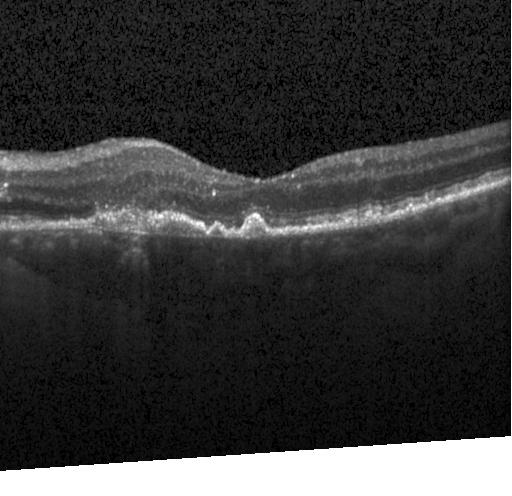
Diagnosis: choroidal neovascularization (CNV).